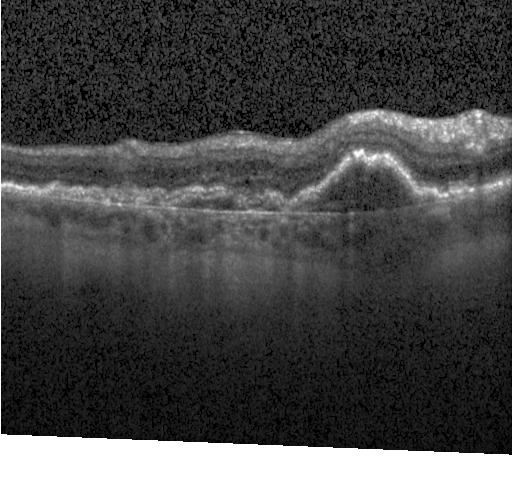
OCT B-scan. Spectral-domain OCT — Diagnosis: CNV.